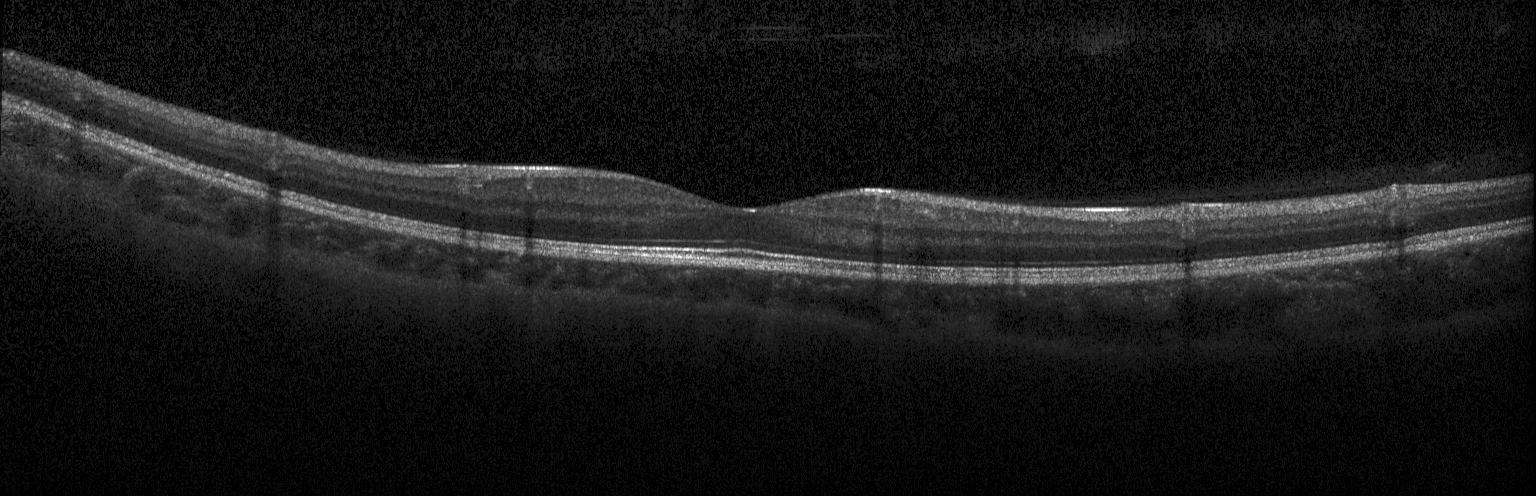
Optical coherence tomography scan — Finding: no choroidal neovascularization, diabetic macular edema, or drusen.